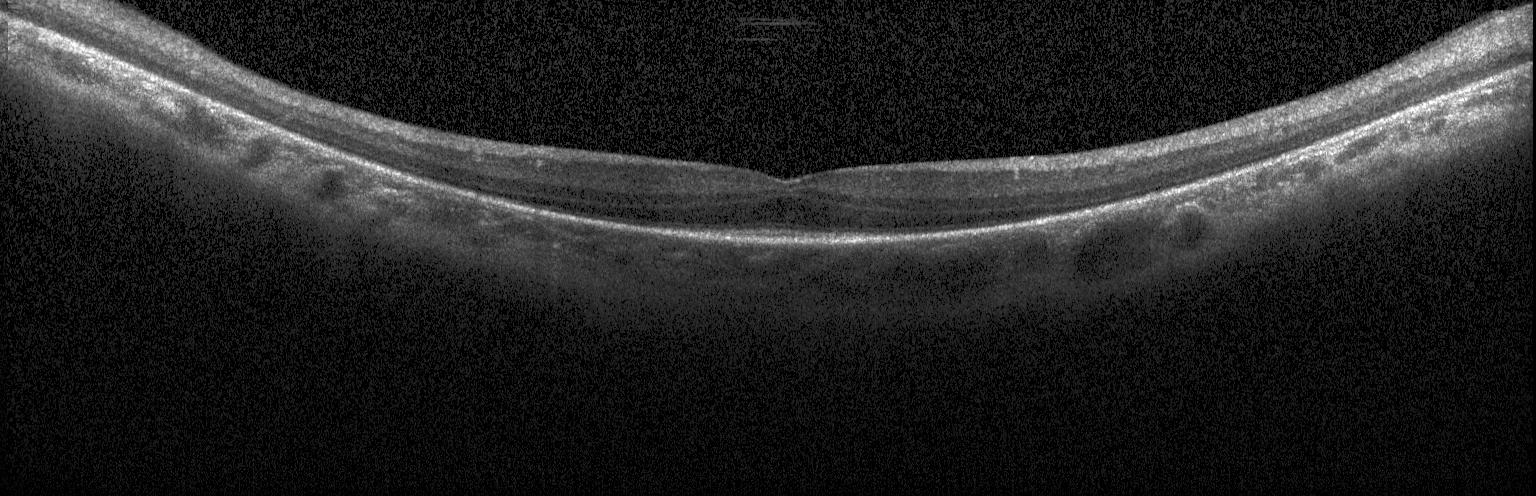
No evidence of CNV, DME, or drusen.